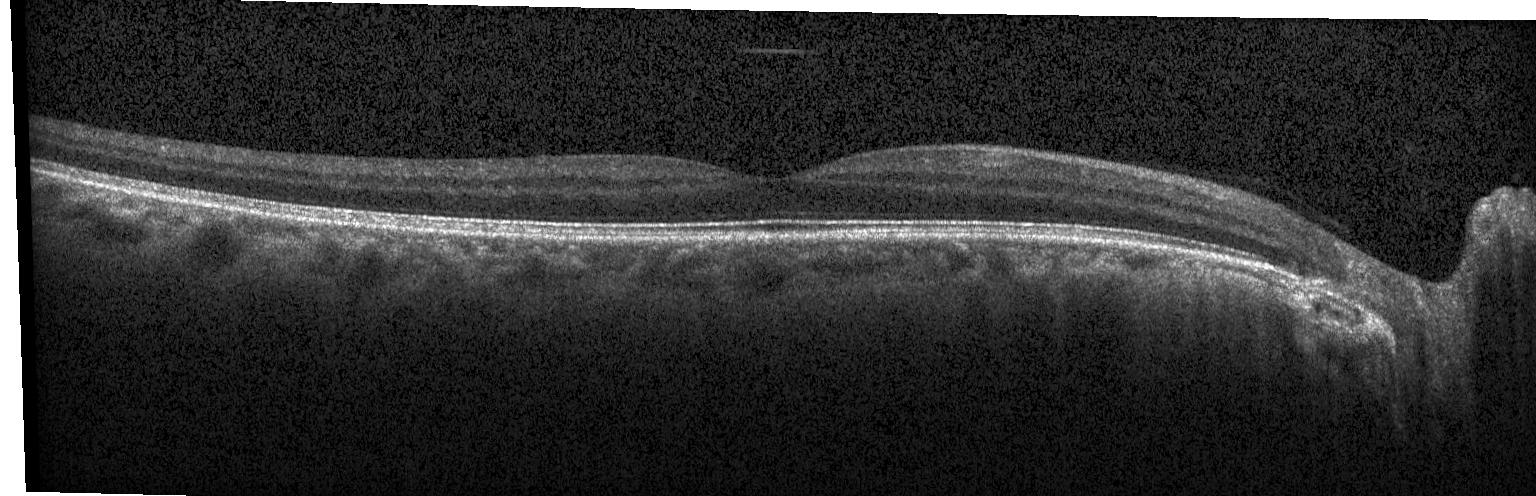

SD-OCT. Retinal OCT cross-section. Instrument: Heidelberg Spectralis. Fovea-centered.
Macular OCT: no evidence of choroidal neovascularization, diabetic macular edema, or drusen.